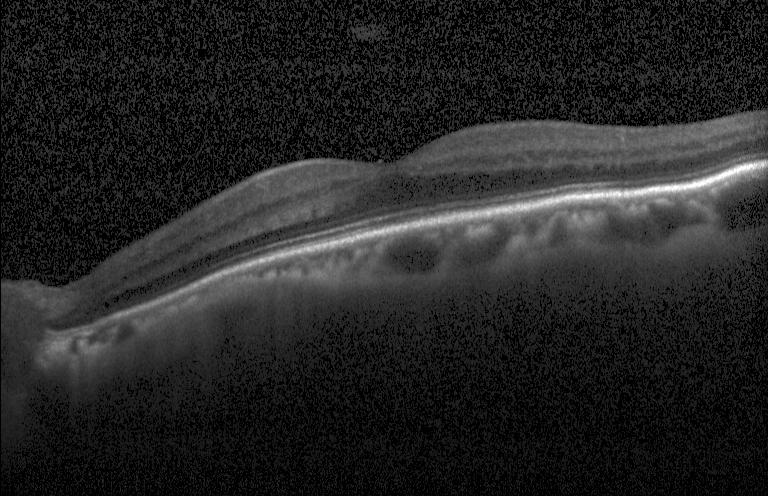
SD-OCT. Retinal OCT B-scan. Acquired on a Heidelberg Spectralis. Through the macula.
This B-scan demonstrates no evidence of choroidal neovascularization, diabetic macular edema, or drusen.